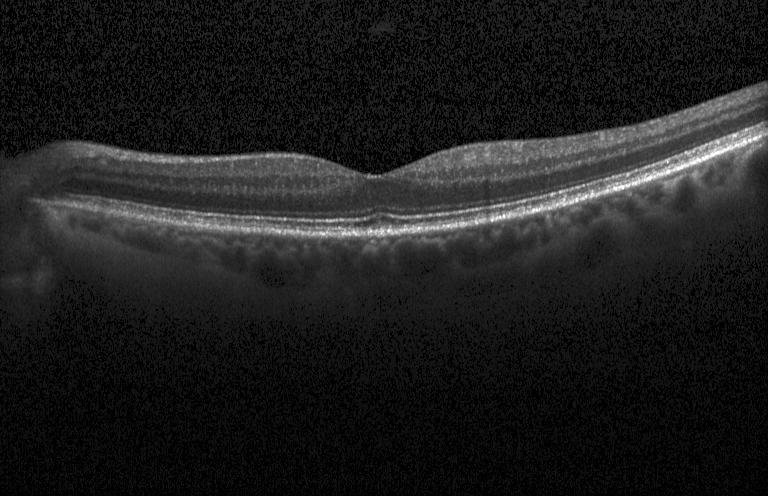 Macular OCT demonstrating no CNV, DME, or drusen.